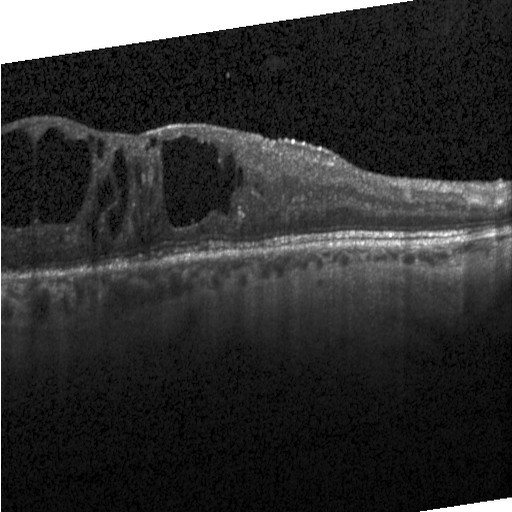 Centered on the fovea, optical coherence tomography scan.
Impression: diabetic macular edema (DME).